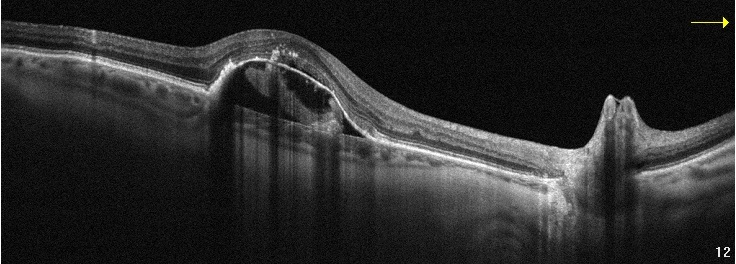 Through the macula, retinal OCT cross-section
Dx: AMD.